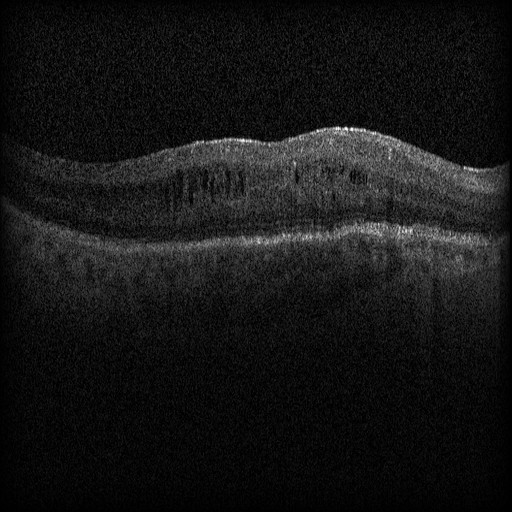

OCT B-scan.
Diagnosis: diabetic macular edema (DME).